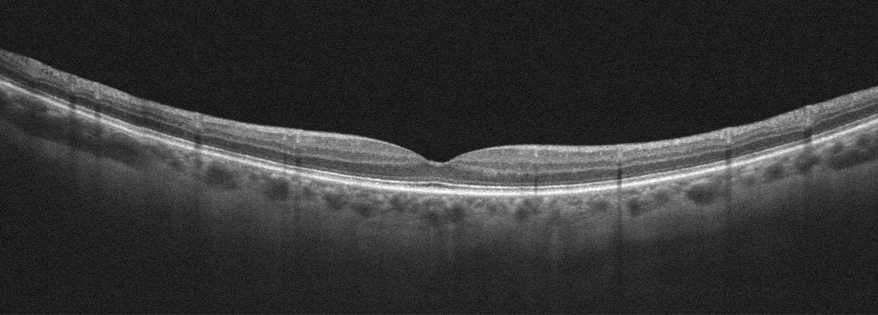

Optical coherence tomography scan
Assessment: no AMD, DME, ERM, RAO, RVO, or VID.